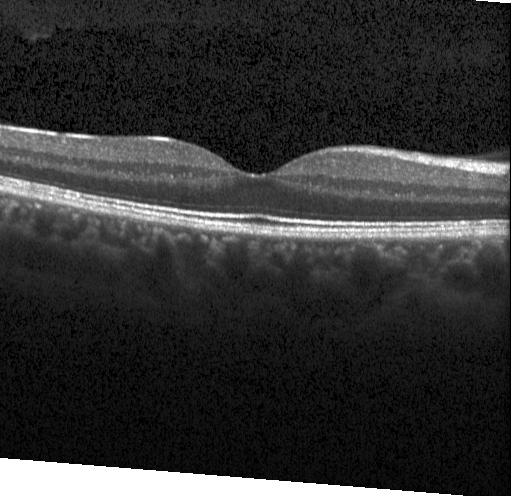
Finding: no choroidal neovascularization, no diabetic macular edema, and no drusen.